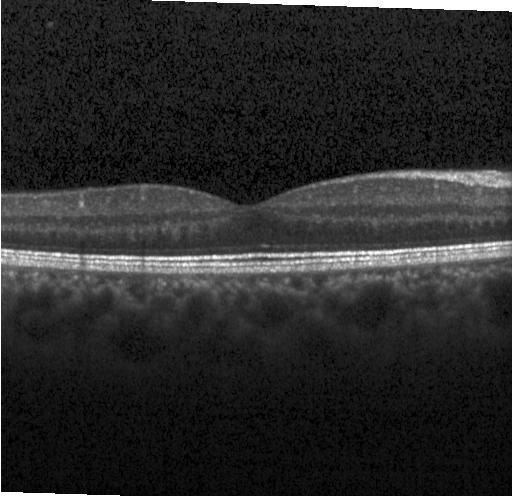
Heidelberg Spectralis, SD-OCT, fovea-centered, OCT B-scan — The scan shows no choroidal neovascularization, diabetic macular edema, or drusen.